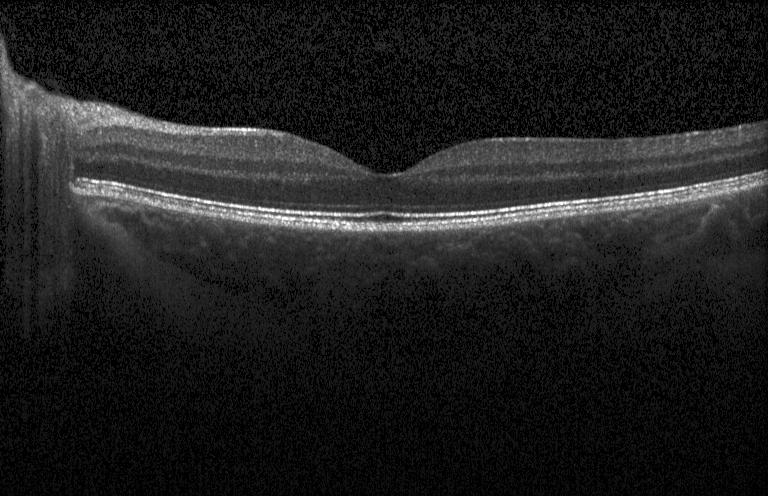 Diagnosis: no choroidal neovascularization, no diabetic macular edema, and no drusen.